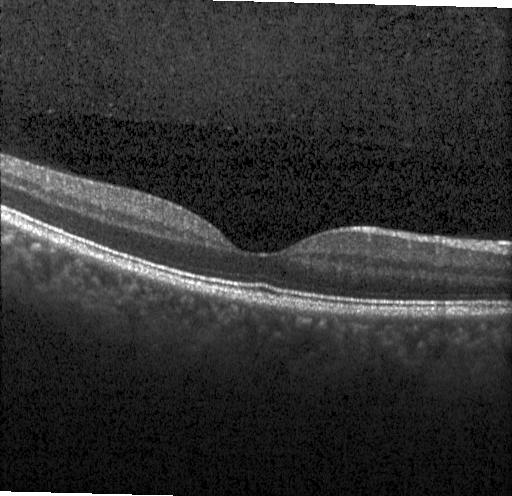 Retinal OCT B-scan.
Impression: no evidence of choroidal neovascularization, diabetic macular edema, or drusen.